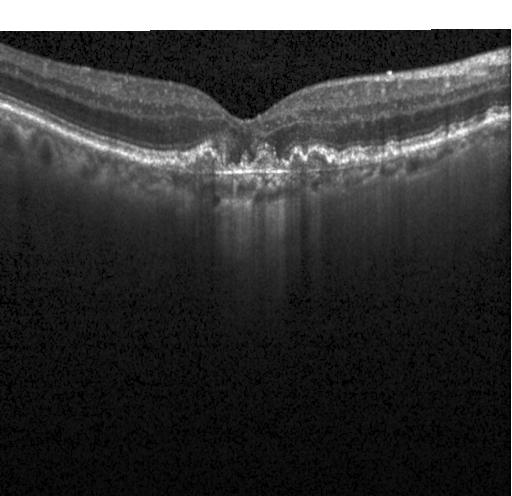

Retinal OCT B-scan — This B-scan demonstrates a choroidal neovascular membrane.